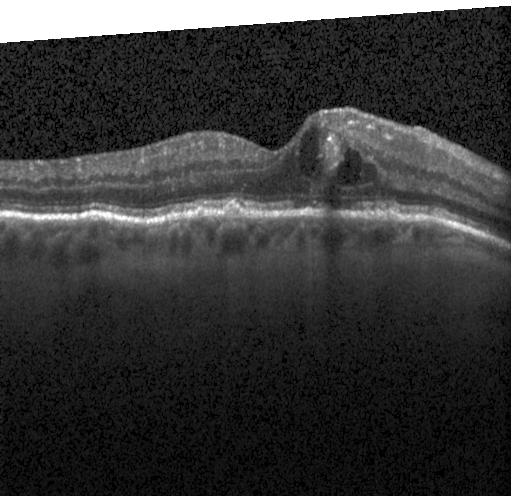
OCT scan showing choroidal neovascularization.